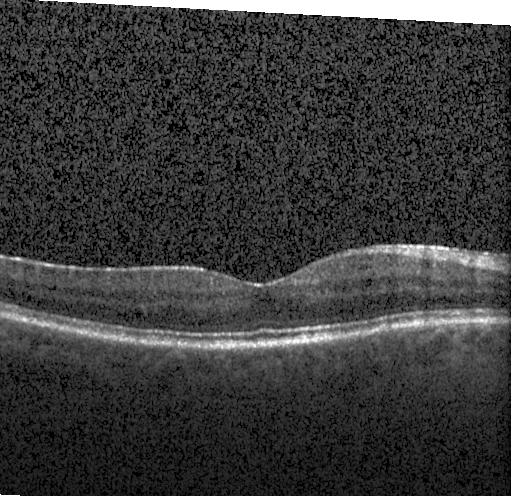 Spectral-domain optical coherence tomography · Heidelberg Spectralis · OCT line scan · centered on the fovea.
No evidence of choroidal neovascularization, diabetic macular edema, or drusen.